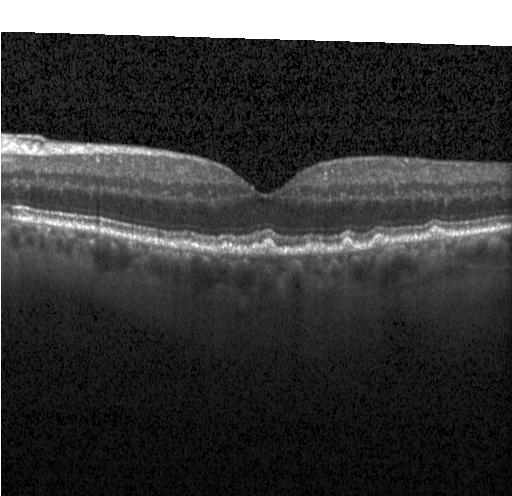
Diagnosis: sub-RPE drusenoid deposits.